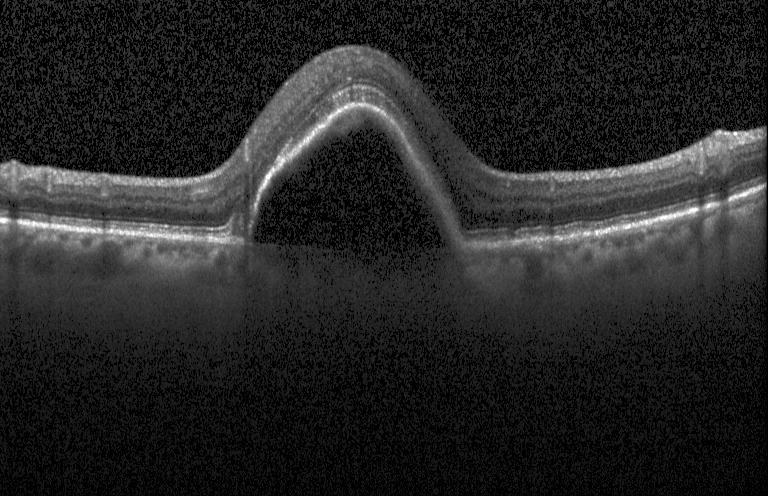
Impression: a choroidal neovascular membrane.